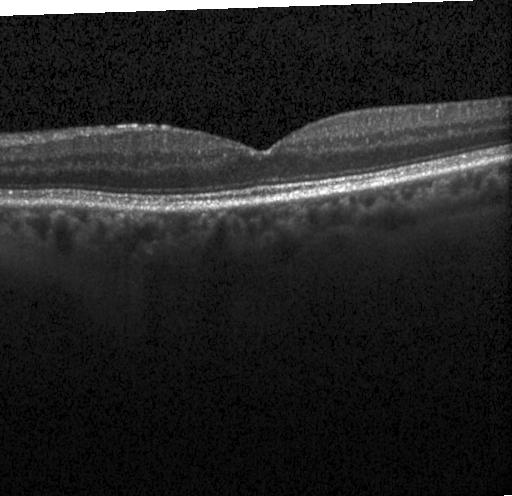

Diagnosis: neither CNV, DME, nor drusen.